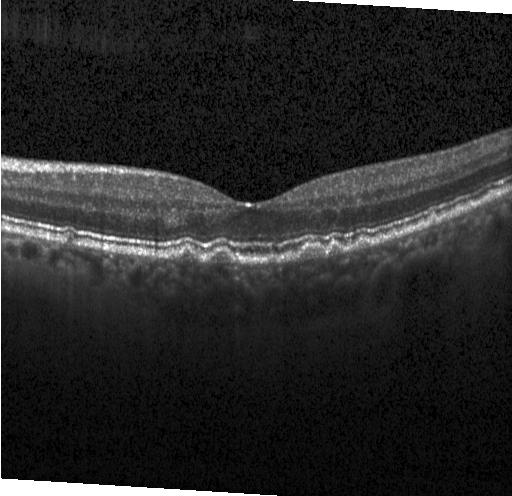
Retinal OCT cross-section
Diagnosis: drusen.